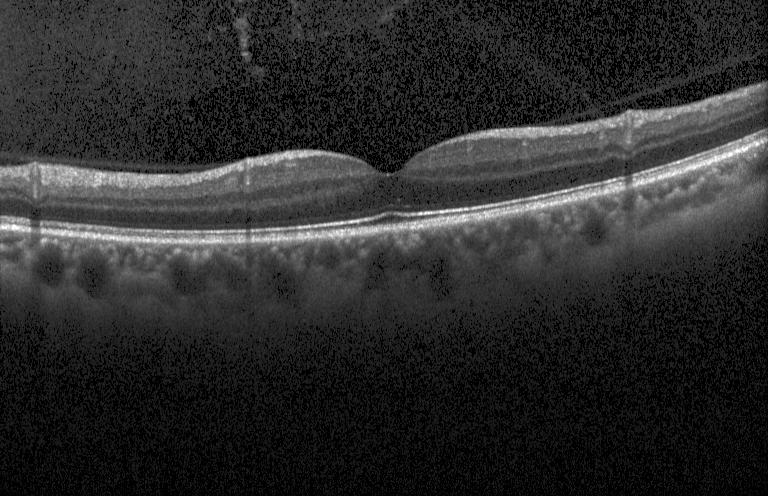 OCT finding: no evidence of choroidal neovascularization, diabetic macular edema, or drusen.